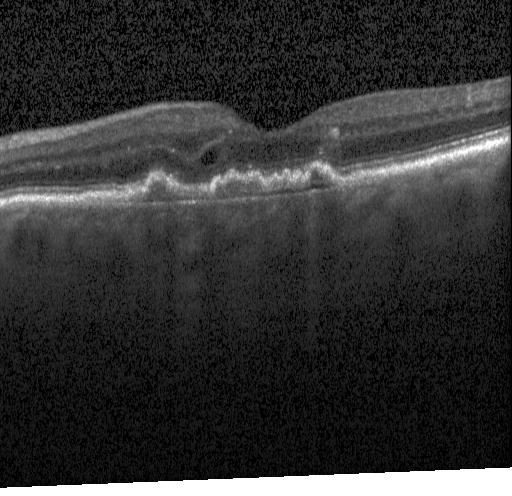 Retinal OCT cross-section.
Impression: a choroidal neovascular membrane.